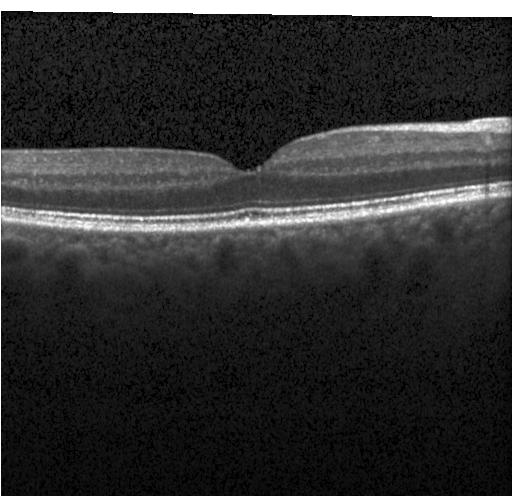

The scan shows no evidence of CNV, DME, or drusen.